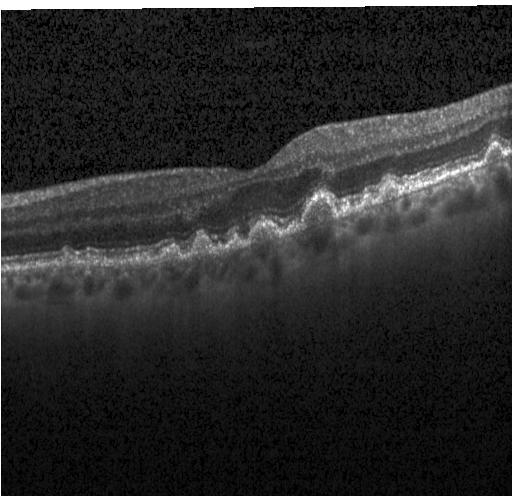 The scan shows sub-RPE drusenoid deposits.